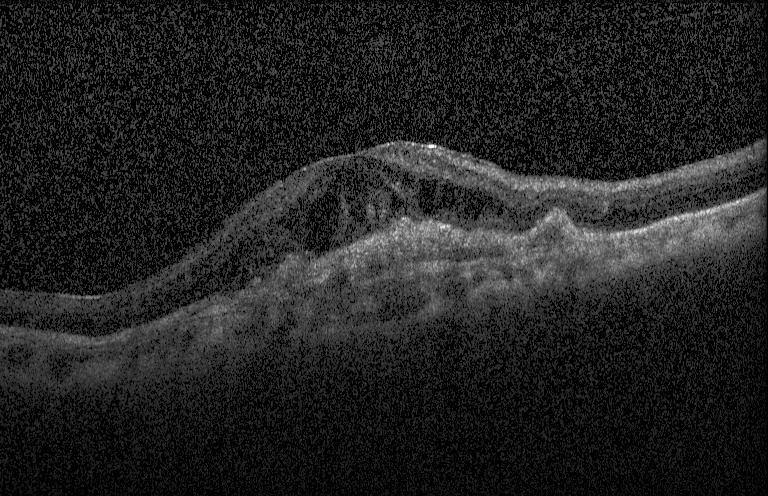
Spectral-domain OCT · instrument: Heidelberg Spectralis · through the macula · OCT line scan.
Finding: a choroidal neovascular membrane.